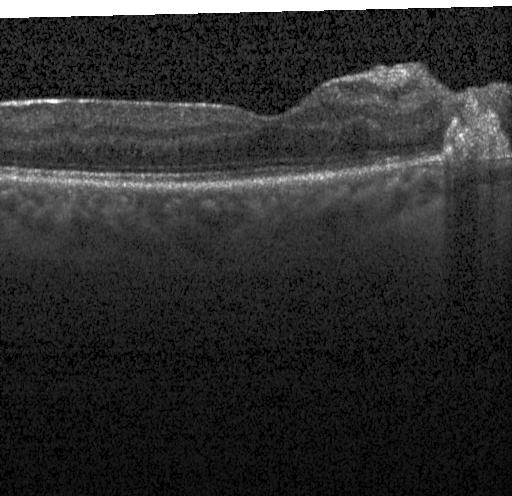

Fovea-centered. Spectral-domain optical coherence tomography. Optical coherence tomography B-scan.
Impression: a choroidal neovascular membrane.